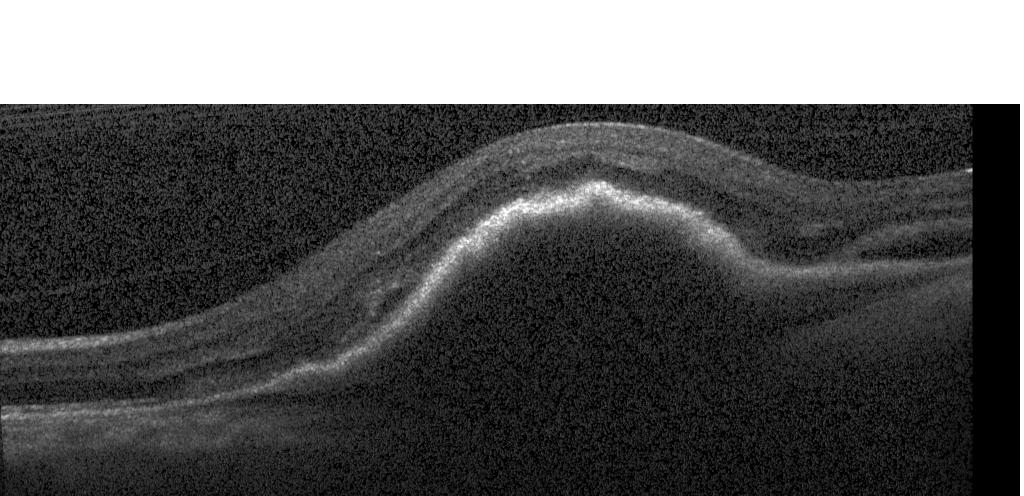

Assessment: choroidal neovascularization.